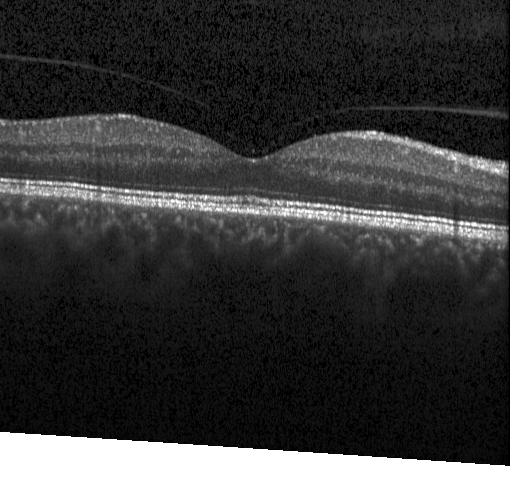

OCT B-scan; spectral-domain OCT; acquired on a Heidelberg Spectralis; horizontal scan through the fovea. Impression: no choroidal neovascularization, diabetic macular edema, or drusen.